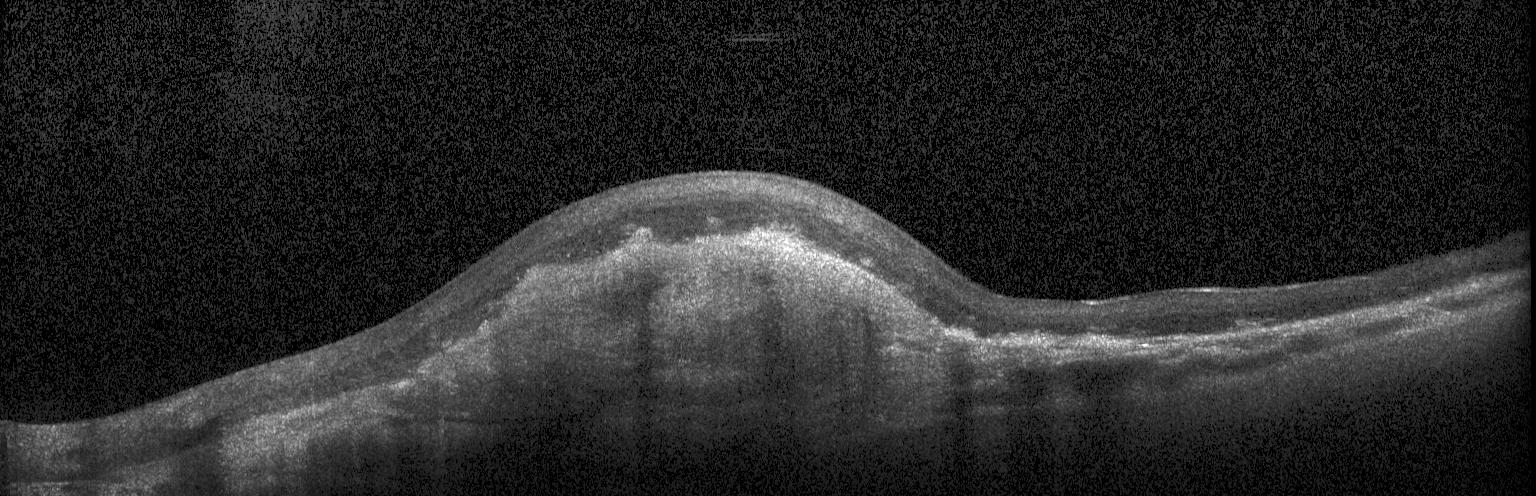

OCT B-scan, Heidelberg Spectralis OCT system, fovea-centered
Impression: a choroidal neovascular membrane.